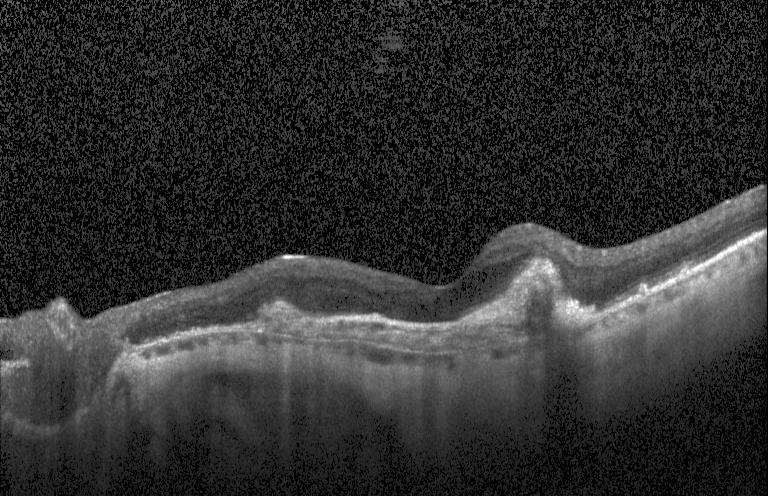

Impression: choroidal neovascularization.